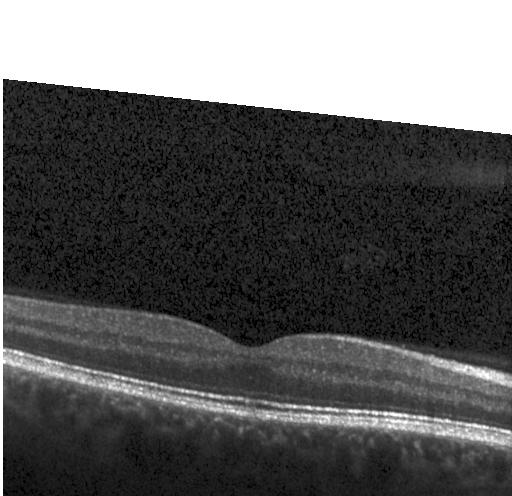
Macular scan · OCT B-scan. Macular OCT: no evidence of choroidal neovascularization, diabetic macular edema, or drusen.